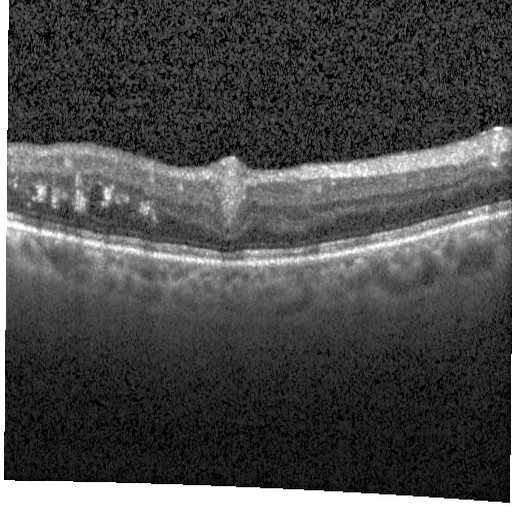
Impression: diabetic macular edema (DME).